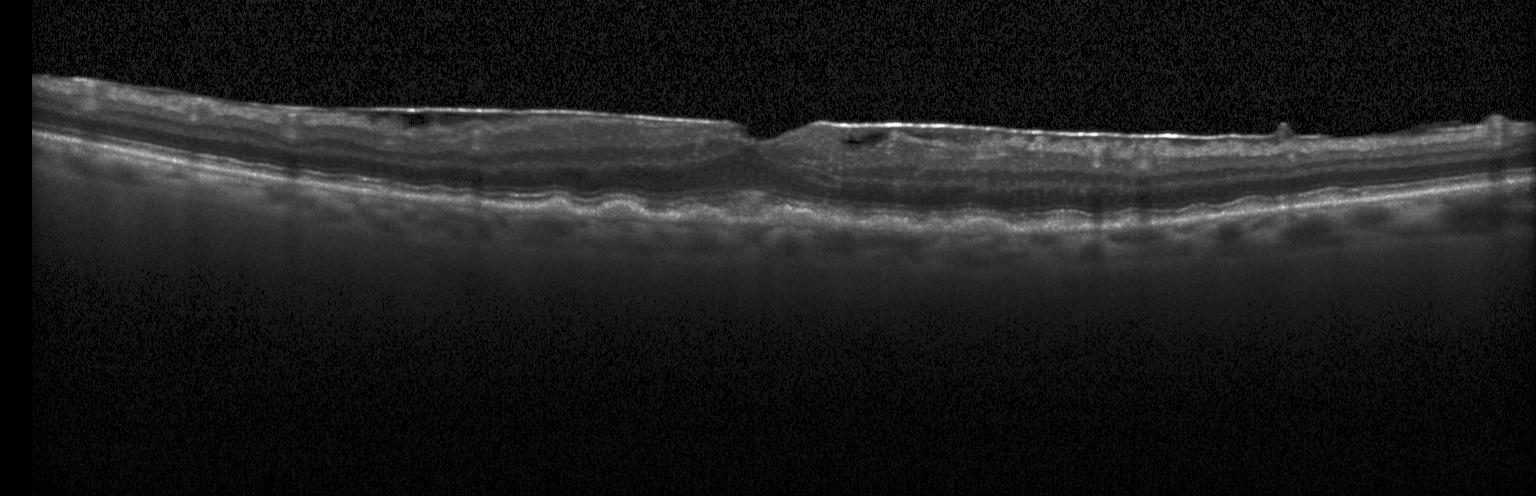

Macular OCT: drusen.